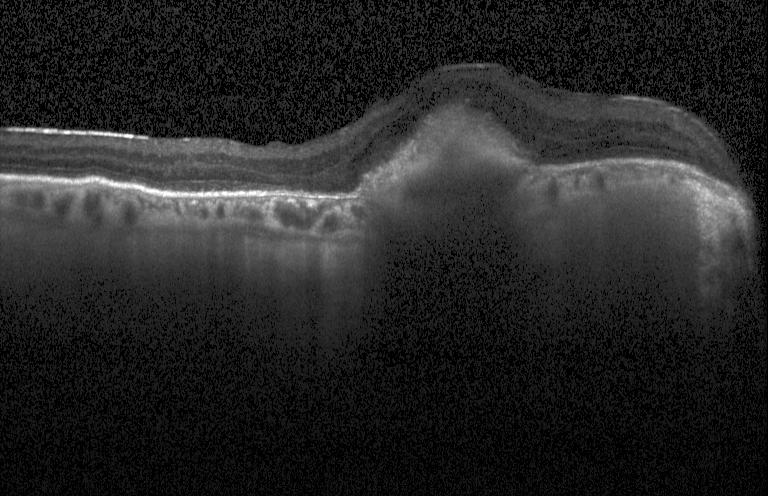
The scan shows a choroidal neovascular membrane.